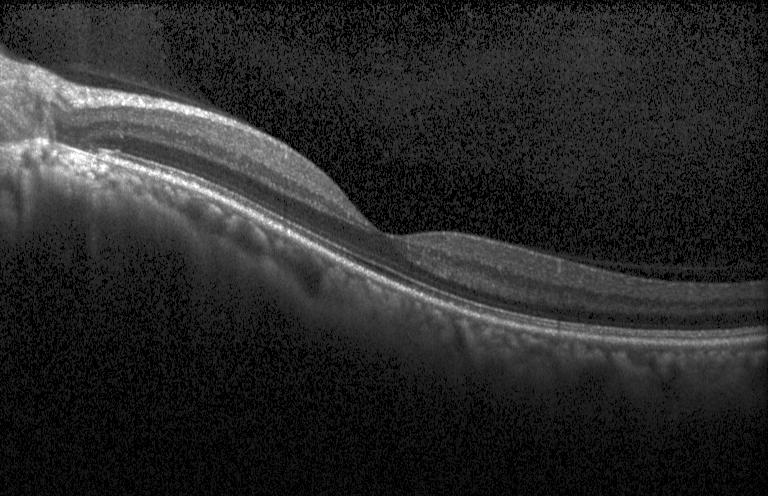

Macular scan; retinal OCT cross-section; spectral-domain OCT; instrument: Heidelberg Spectralis — OCT finding: no evidence of choroidal neovascularization, diabetic macular edema, or drusen.